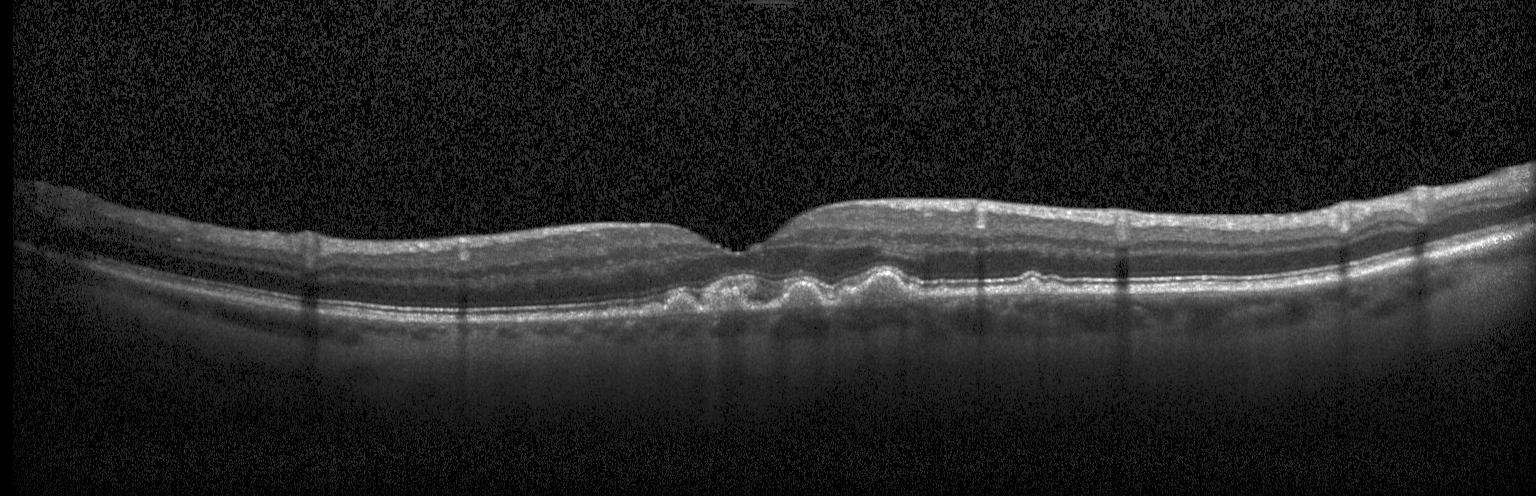

Retinal OCT B-scan
Dx: sub-RPE drusenoid deposits.